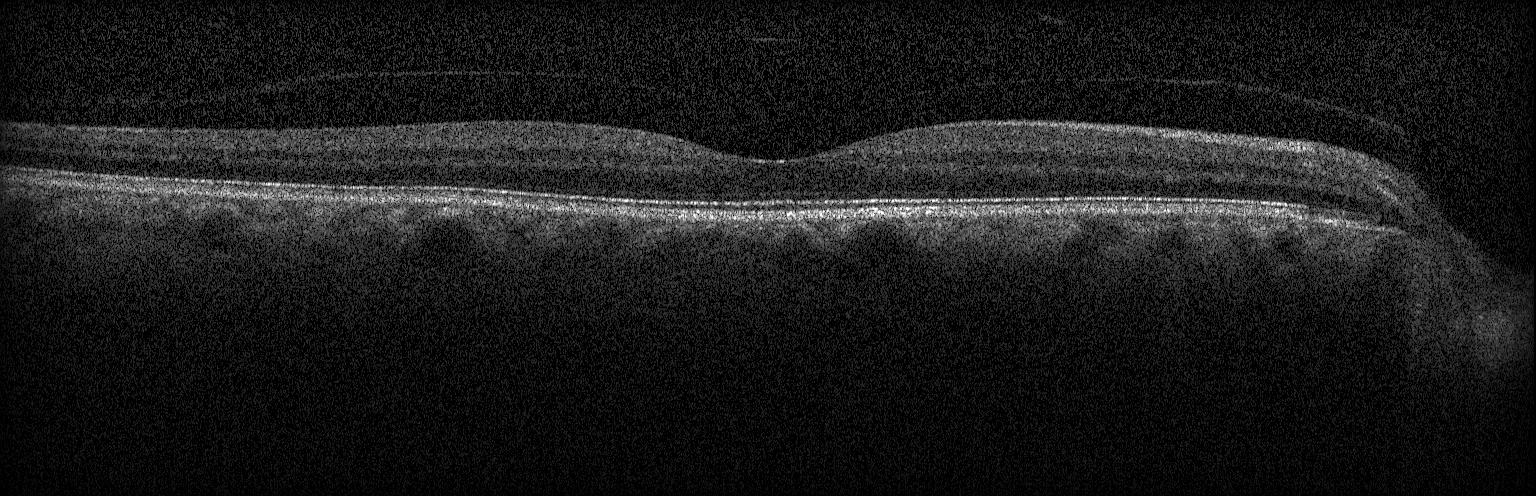
Heidelberg Spectralis · OCT B-scan · spectral-domain optical coherence tomography — Impression: no choroidal neovascularization, no diabetic macular edema, and no drusen.